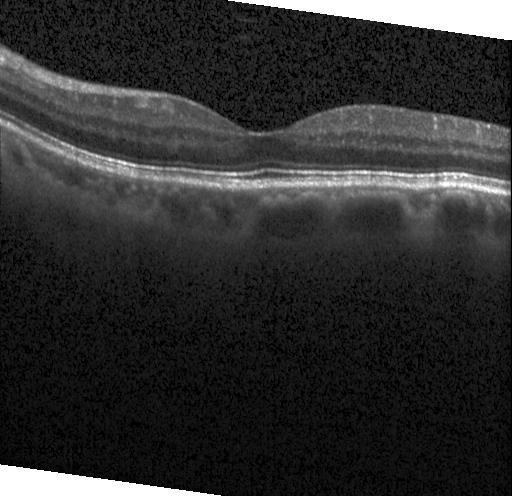

OCT line scan.
No choroidal neovascularization, diabetic macular edema, or drusen.